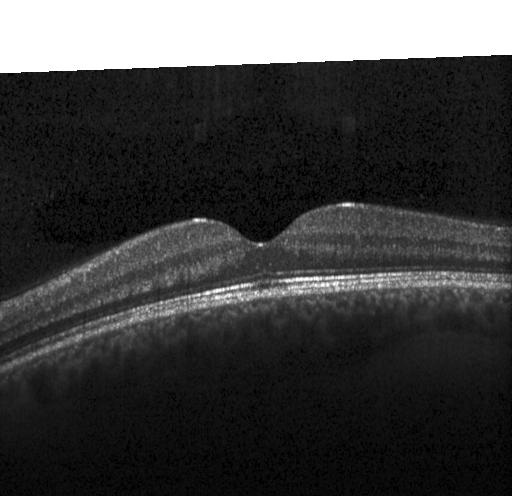
OCT line scan
Diagnosis: no CNV, DME, or drusen.